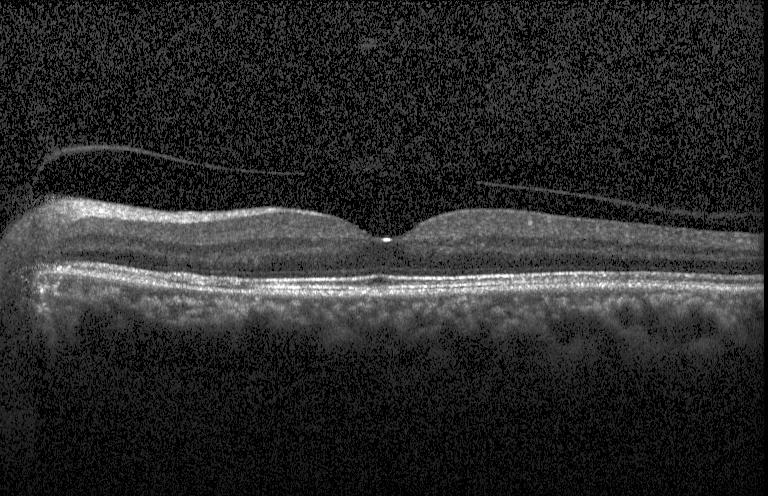
Heidelberg Spectralis. Spectral-domain OCT. OCT B-scan. Fovea-centered
Assessment: neither choroidal neovascularization, diabetic macular edema, nor drusen.